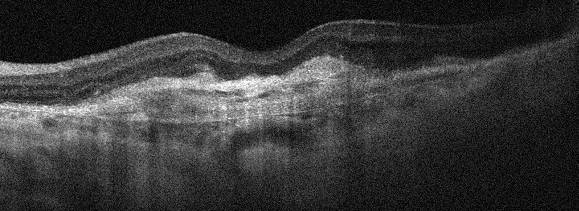
Retinal OCT B-scan, macular scan, left eye.
Finding: age-related macular degeneration (AMD).